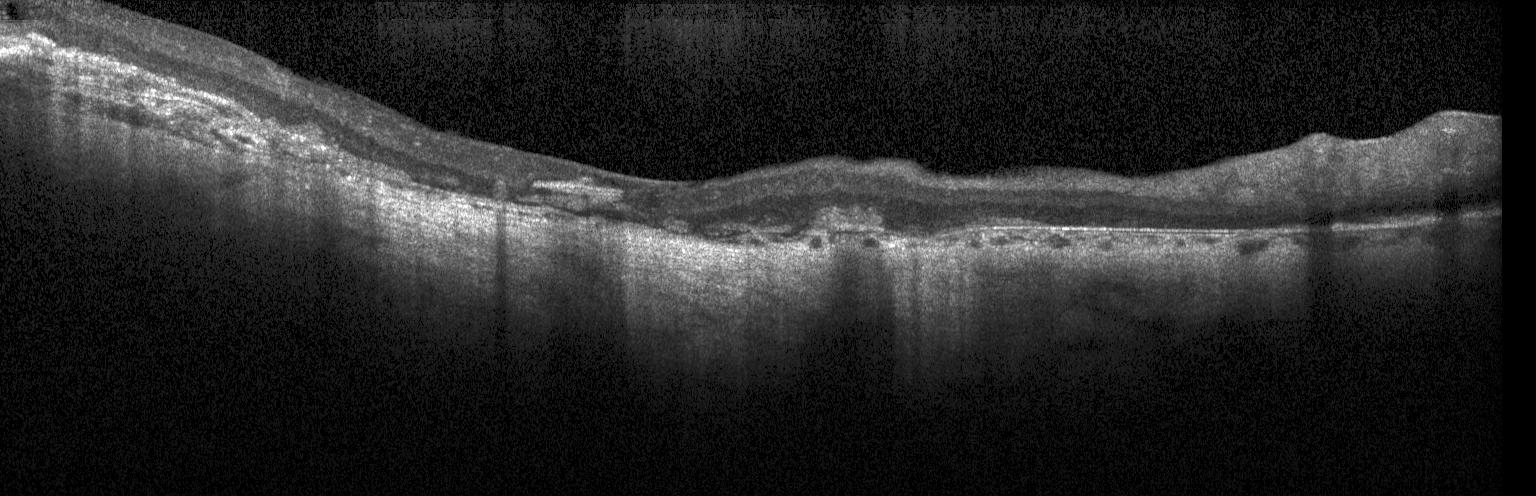
Retinal OCT B-scan
Diagnosis: a choroidal neovascular membrane.